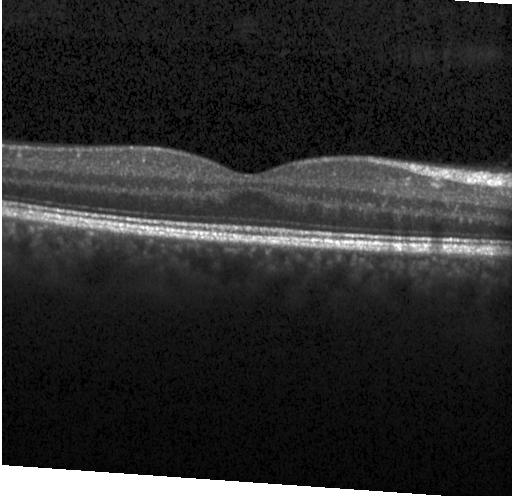
The scan shows no evidence of choroidal neovascularization, diabetic macular edema, or drusen.